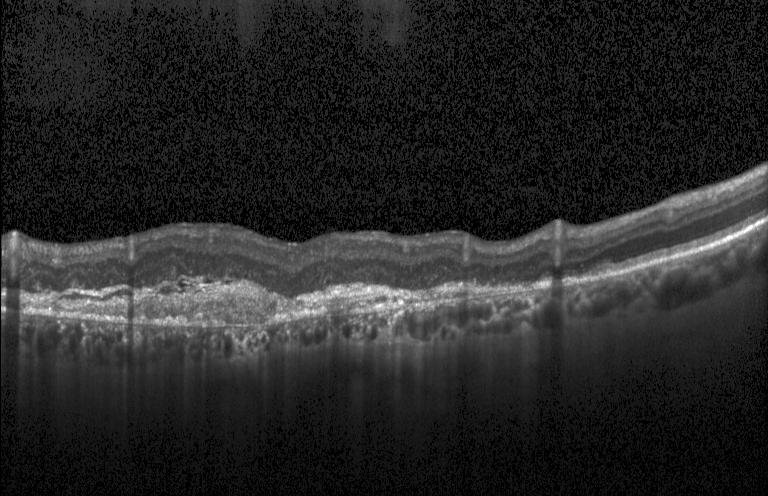 SD-OCT; Heidelberg Spectralis OCT system; horizontal scan through the fovea; optical coherence tomography scan. Impression: choroidal neovascularization.